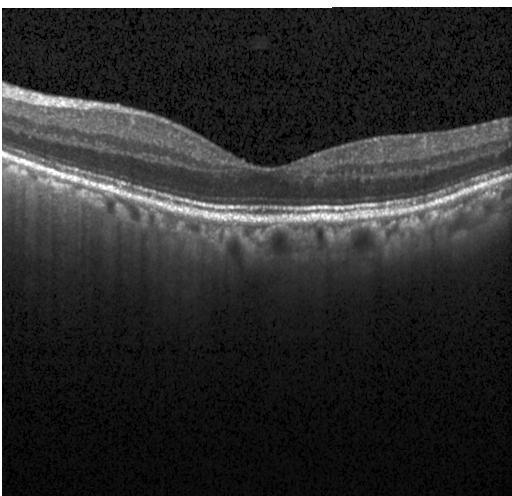
Heidelberg Spectralis OCT system; spectral-domain optical coherence tomography; optical coherence tomography B-scan — The scan shows neither choroidal neovascularization, diabetic macular edema, nor drusen.